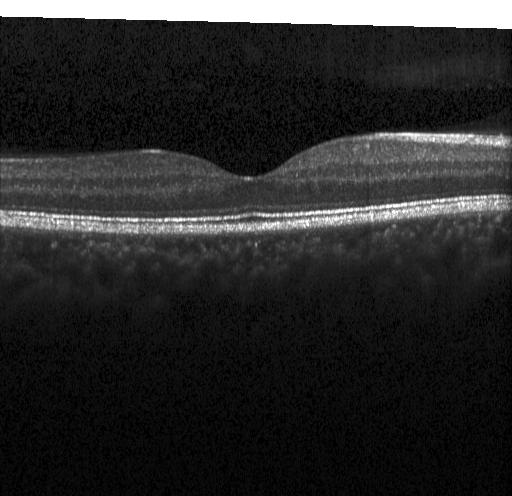
OCT scan showing no choroidal neovascularization, no diabetic macular edema, and no drusen.